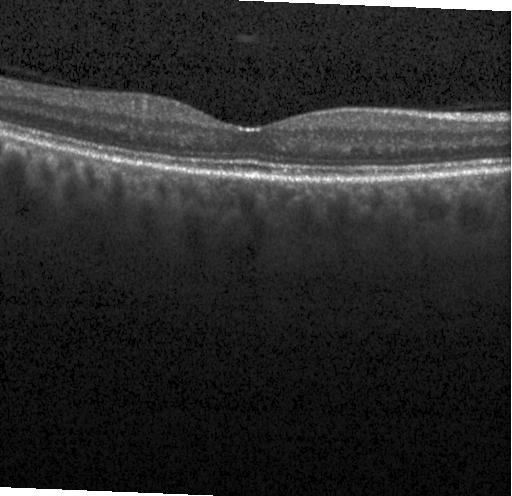

Horizontal scan through the fovea; Heidelberg Spectralis OCT system; optical coherence tomography B-scan; SD-OCT.
Diagnosis: no evidence of choroidal neovascularization, diabetic macular edema, or drusen.